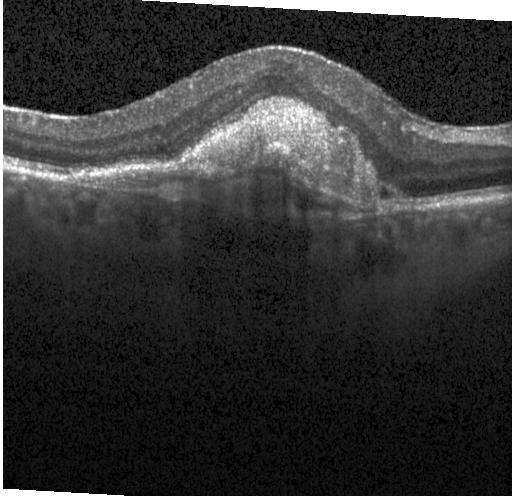 Optical coherence tomography scan · Heidelberg Spectralis · through the macula · spectral-domain OCT.
CNV.